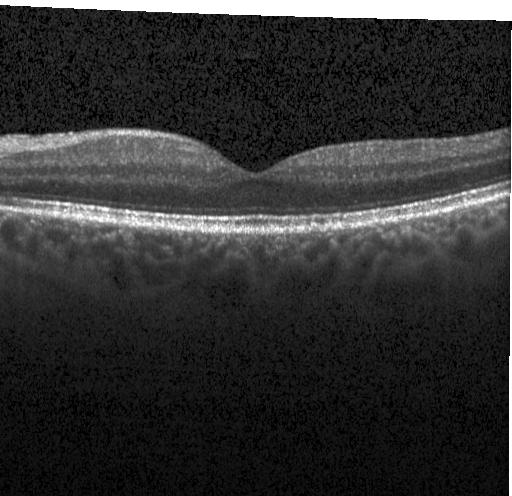

Macular OCT: no choroidal neovascularization, no diabetic macular edema, and no drusen.